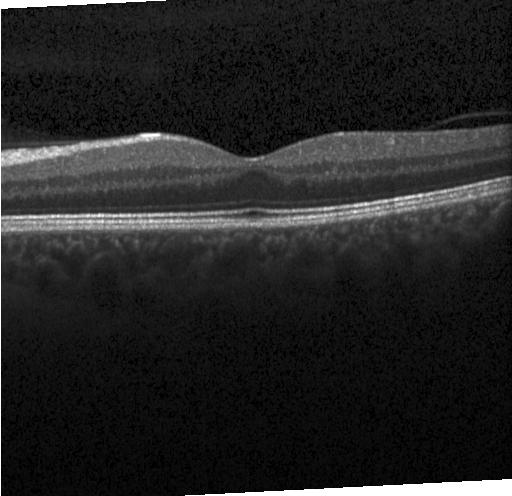

Spectral-domain optical coherence tomography. Optical coherence tomography scan. Heidelberg Spectralis OCT system. Macular scan — Dx: no choroidal neovascularization, diabetic macular edema, or drusen.